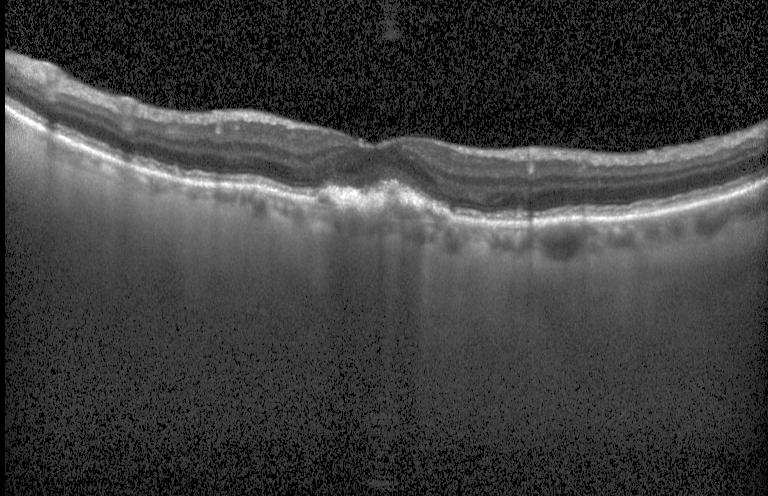

Heidelberg Spectralis. Spectral-domain OCT. Through the macula. Retinal OCT B-scan
Impression: a choroidal neovascular membrane.